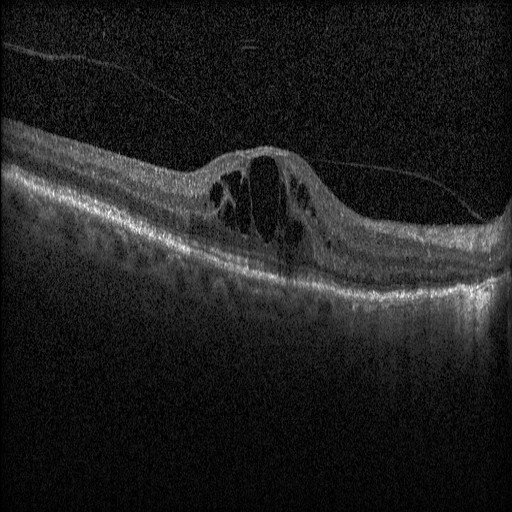 OCT line scan; spectral-domain OCT — Finding: DME.